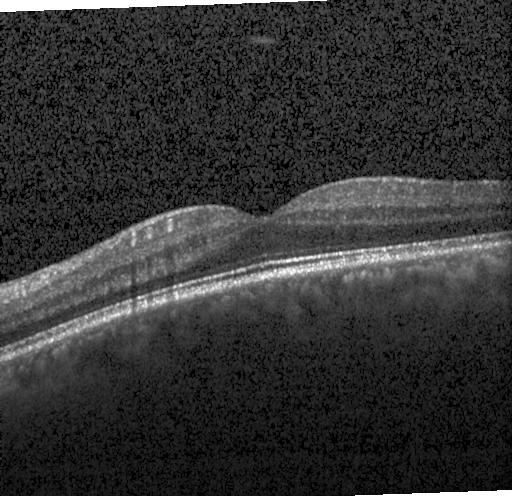
Retinal OCT cross-section.
Finding: no evidence of CNV, DME, or drusen.